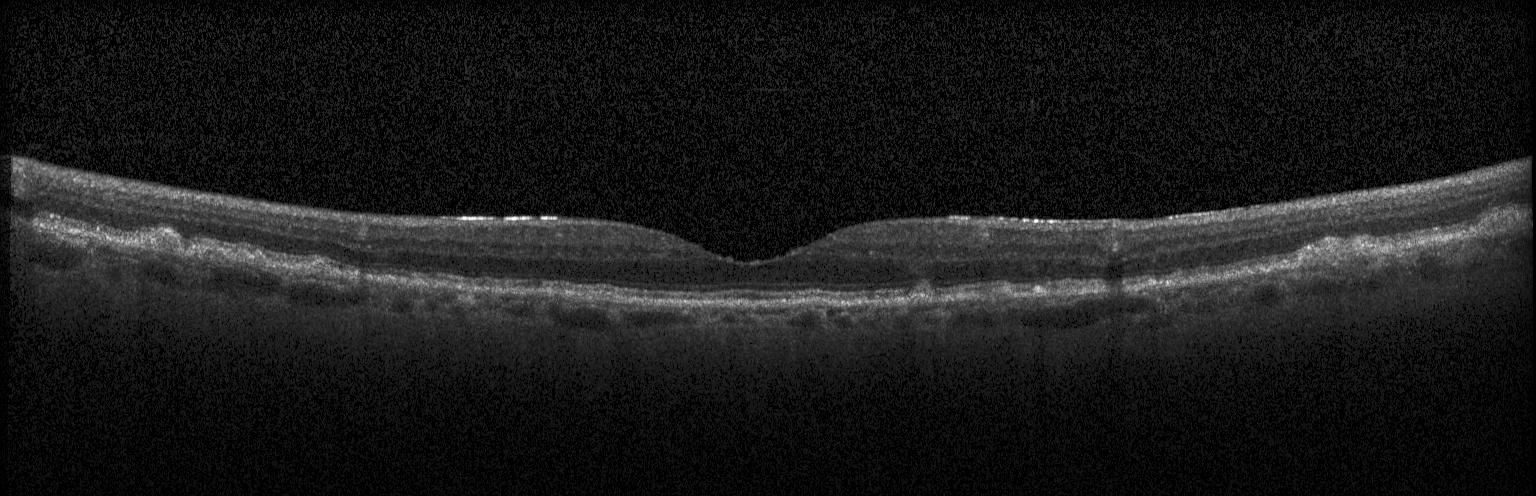

OCT B-scan showing sub-RPE drusenoid deposits.